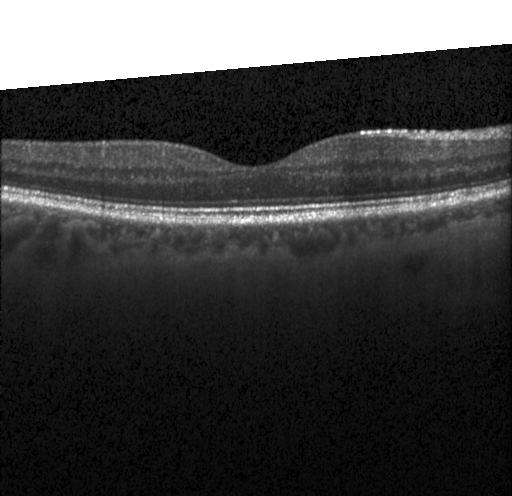 OCT B-scan.
Finding: no choroidal neovascularization, diabetic macular edema, or drusen.